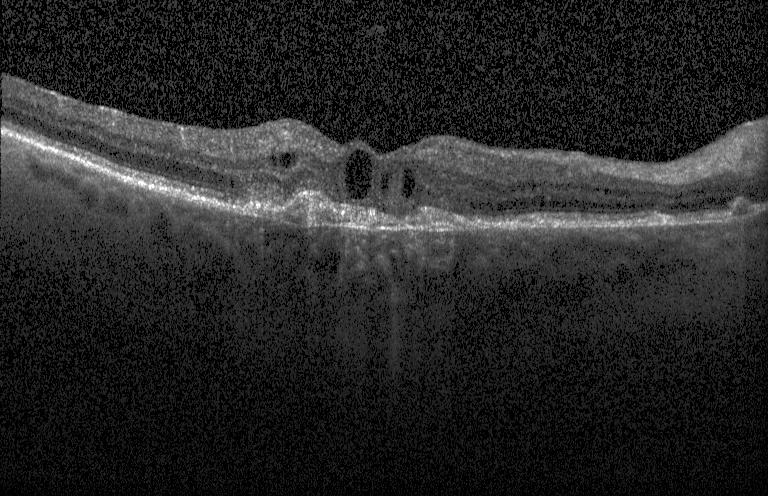

Fovea-centered · retinal OCT B-scan · Heidelberg Spectralis OCT system
Finding: a choroidal neovascular membrane.